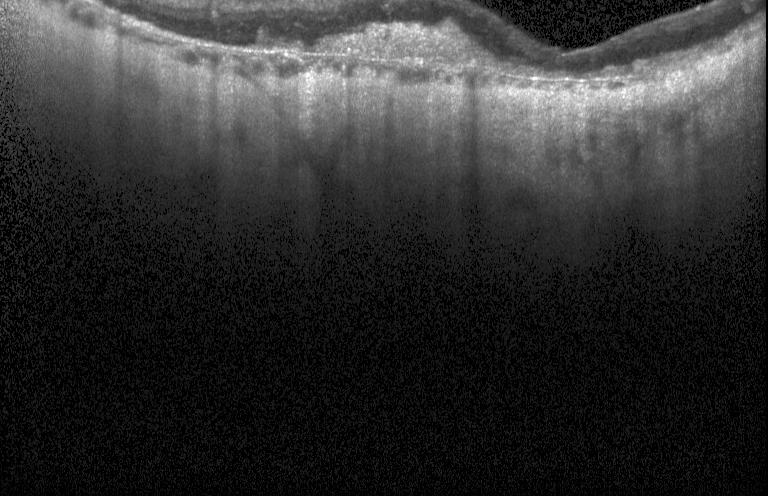 OCT B-scan showing choroidal neovascularization (CNV).